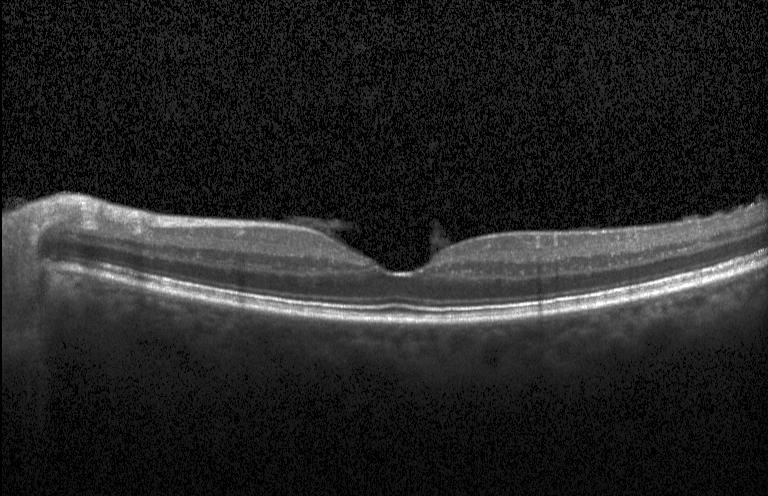 Retinal OCT cross-section · spectral-domain optical coherence tomography.
Finding: no evidence of CNV, DME, or drusen.